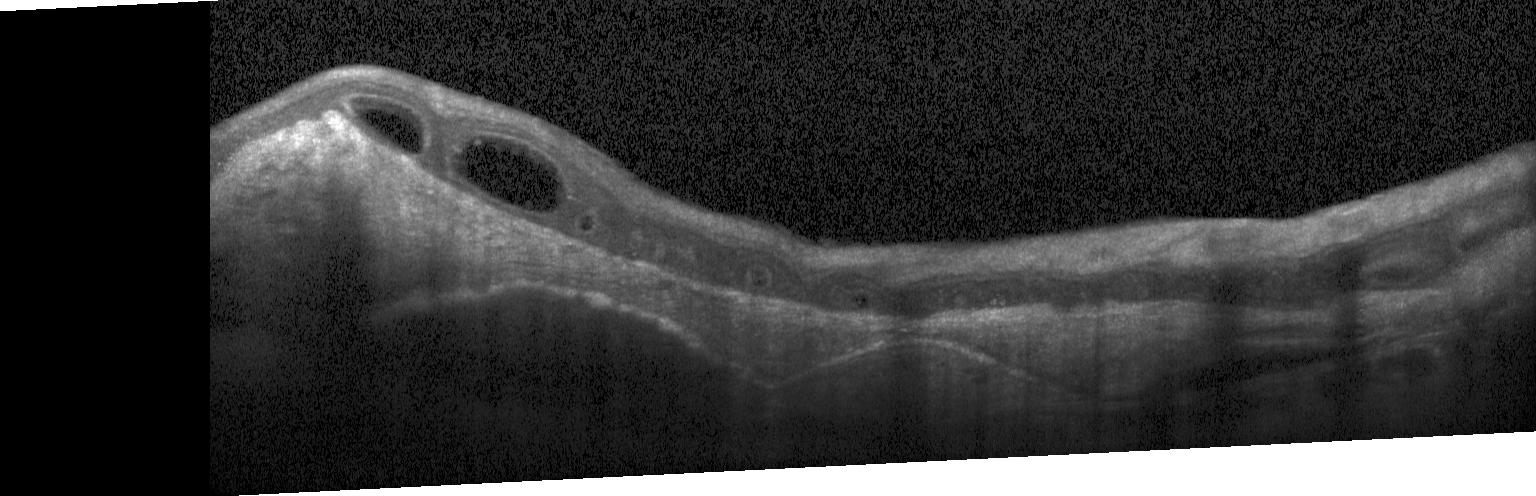

Retinal OCT B-scan.
Dx: a choroidal neovascular membrane.